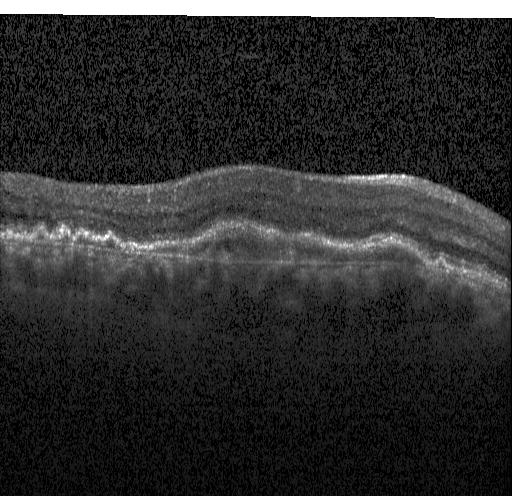 Dx: a choroidal neovascular membrane.